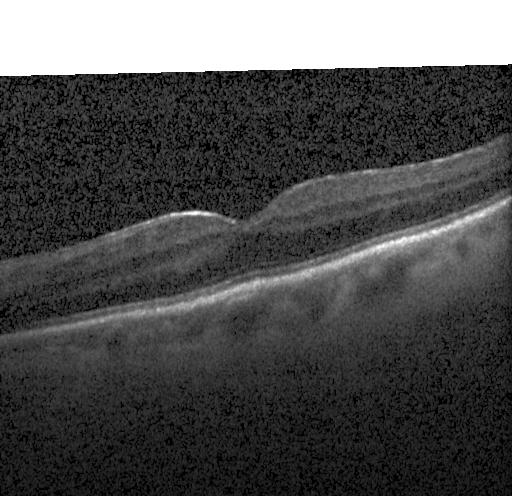
Retinal OCT B-scan.
Diagnosis: no CNV, DME, or drusen.